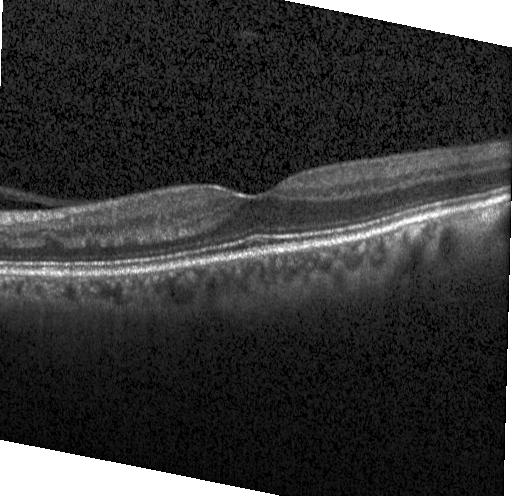 Diagnosis: no evidence of CNV, DME, or drusen.